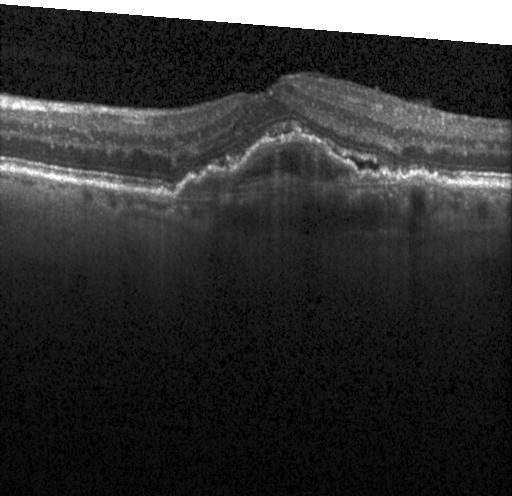

Macular OCT demonstrating CNV.